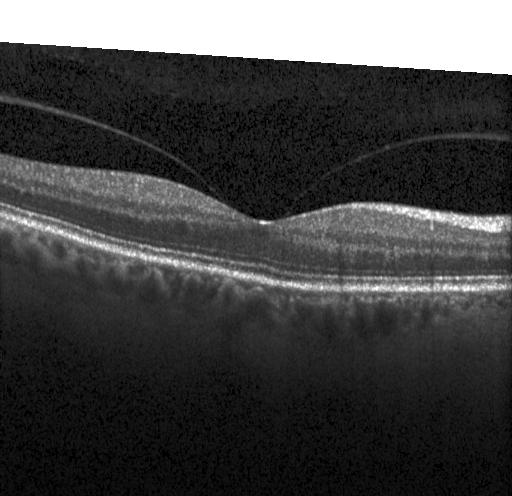

OCT B-scan showing no evidence of CNV, DME, or drusen.